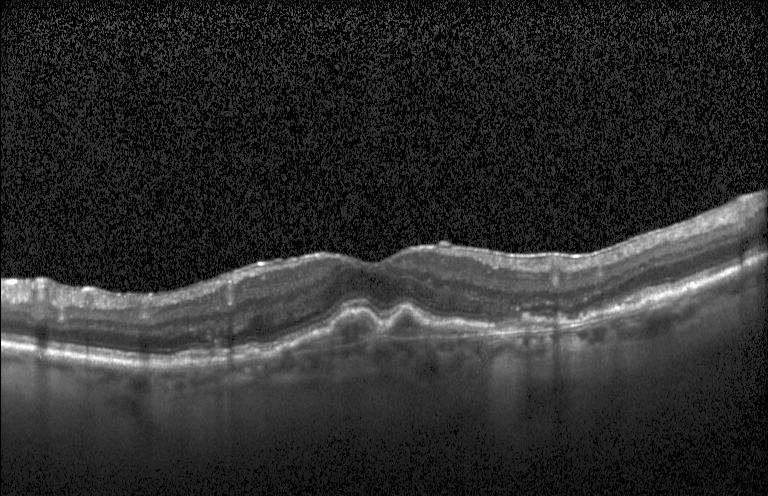

Impression: choroidal neovascularization (CNV).